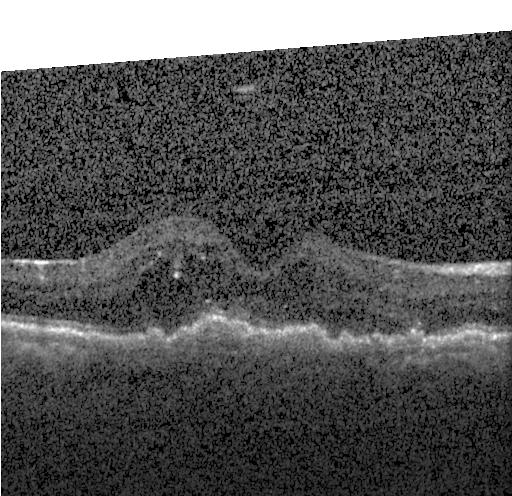 SD-OCT. Fovea-centered. Optical coherence tomography B-scan. Instrument: Heidelberg Spectralis. Assessment: CNV.